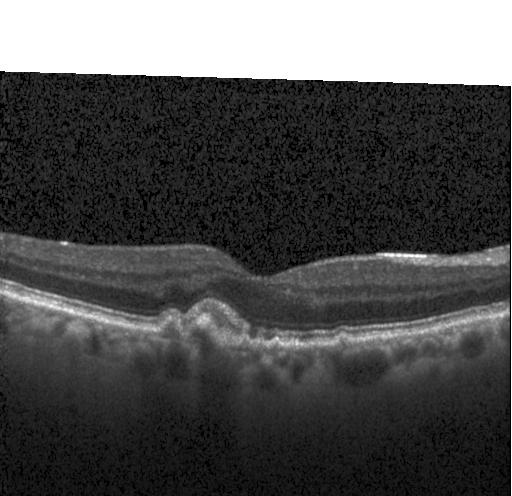 OCT B-scan; acquired on a Heidelberg Spectralis.
Assessment: a choroidal neovascular membrane.